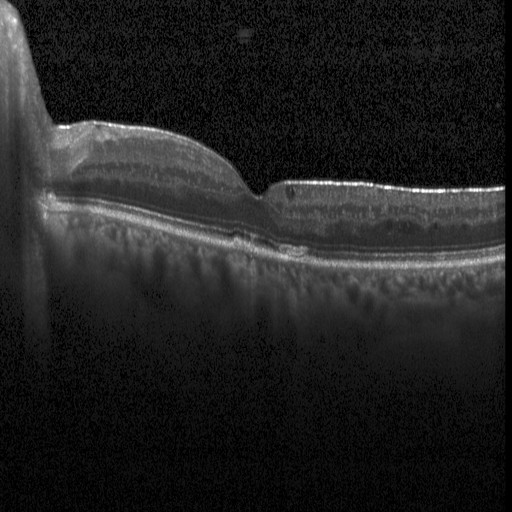 Heidelberg Spectralis; through the macula; retinal OCT cross-section
Dx: DME.